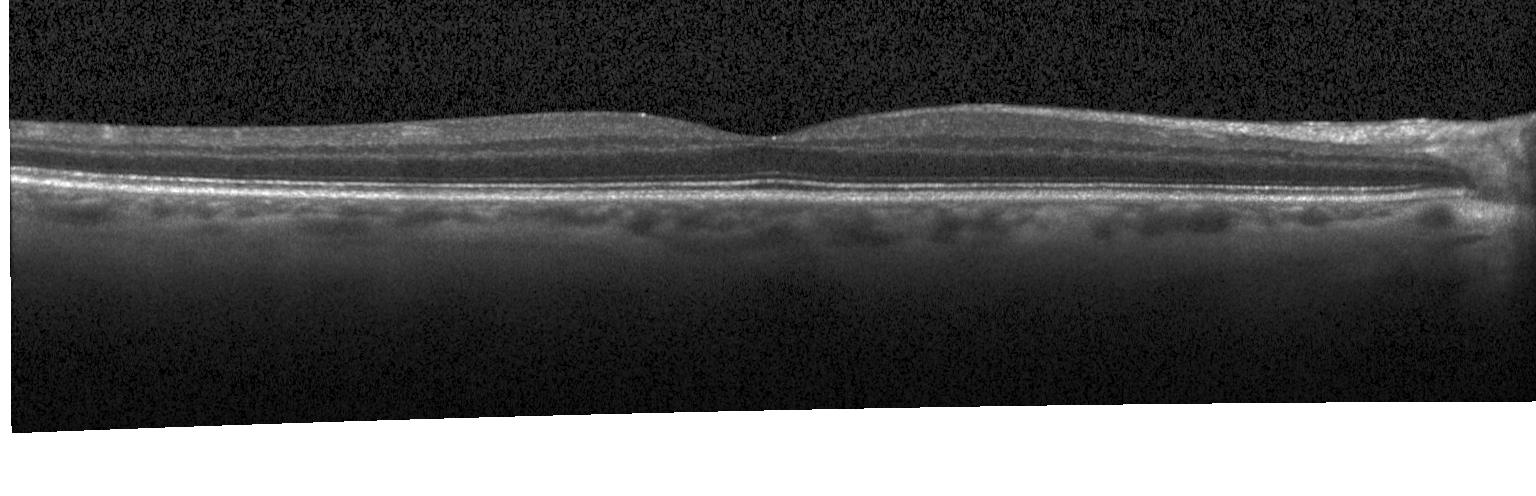 Optical coherence tomography B-scan.
Impression: neither CNV, DME, nor drusen.